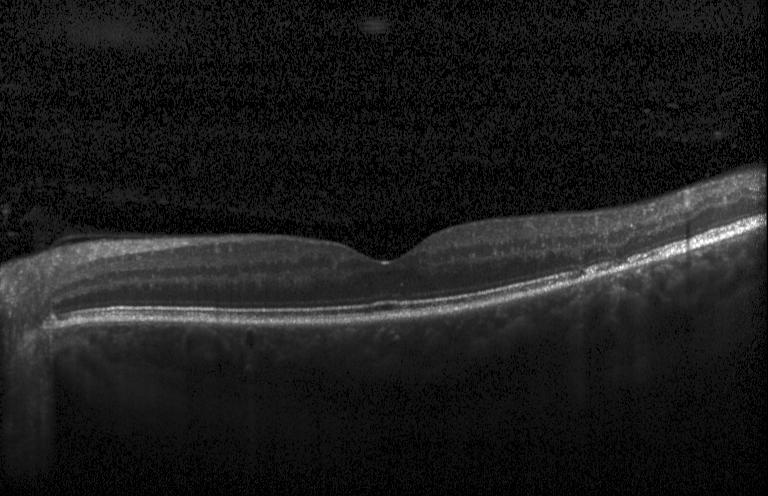 Impression: neither CNV, DME, nor drusen.